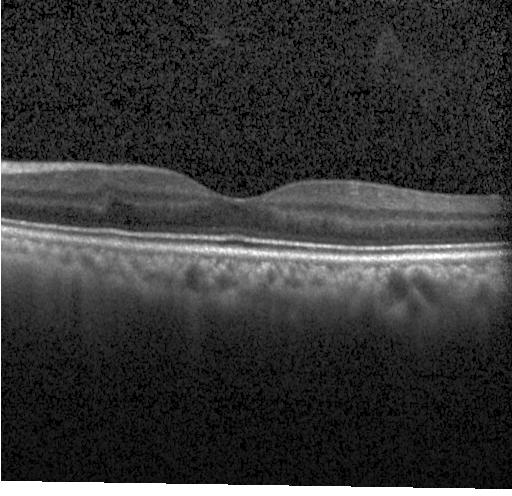
OCT scan showing no choroidal neovascularization, diabetic macular edema, or drusen.